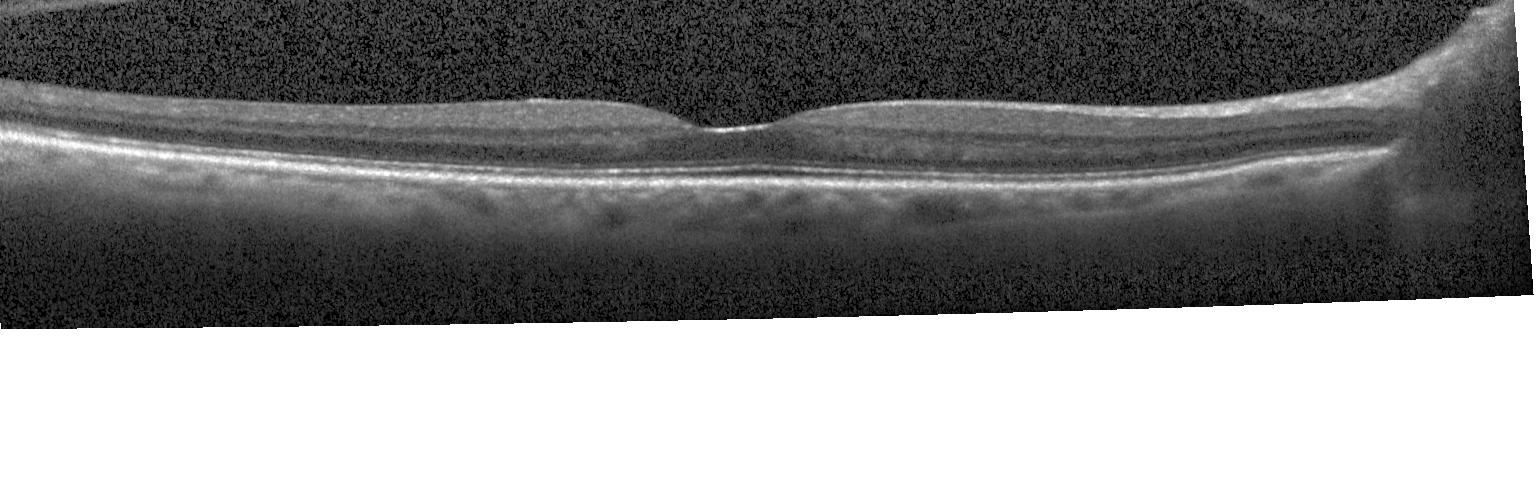 Finding: neither choroidal neovascularization, diabetic macular edema, nor drusen.